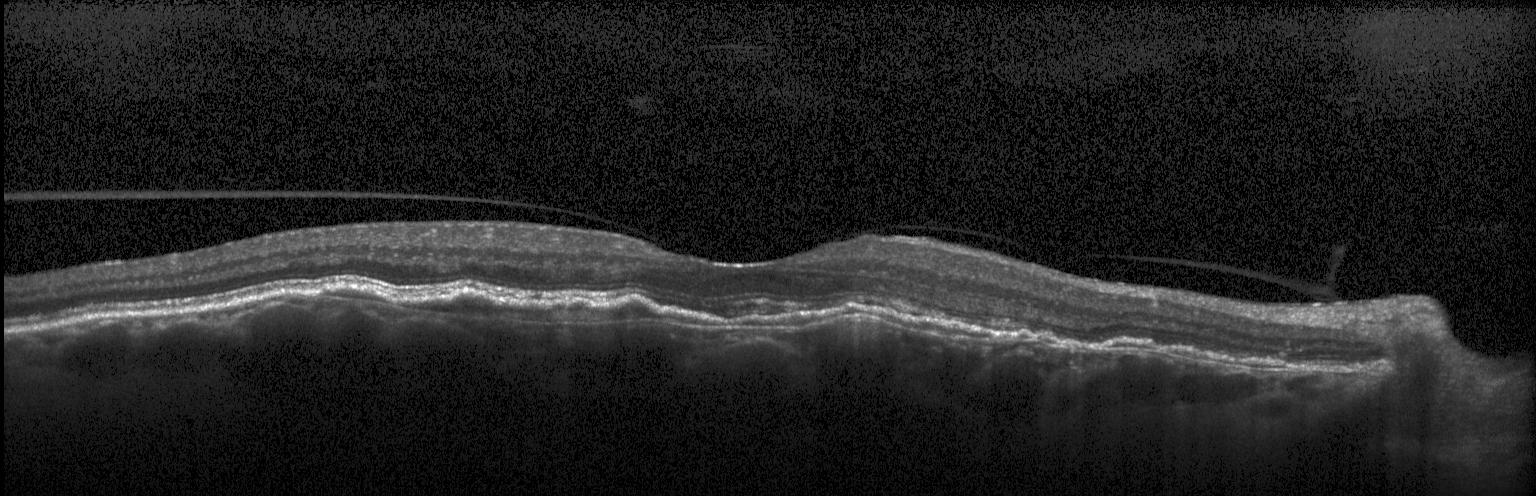
OCT B-scan — Finding: choroidal neovascularization (CNV).